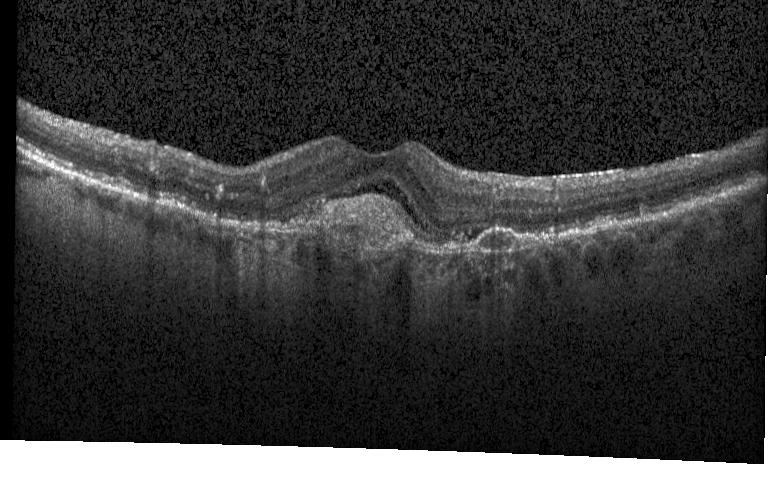 Diagnosis: choroidal neovascularization (CNV).